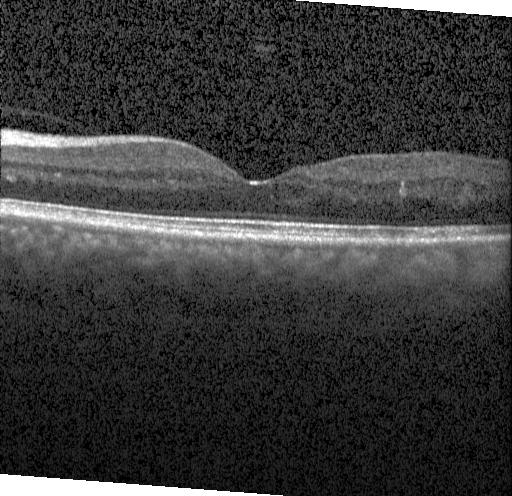

Optical coherence tomography B-scan — Assessment: DME.